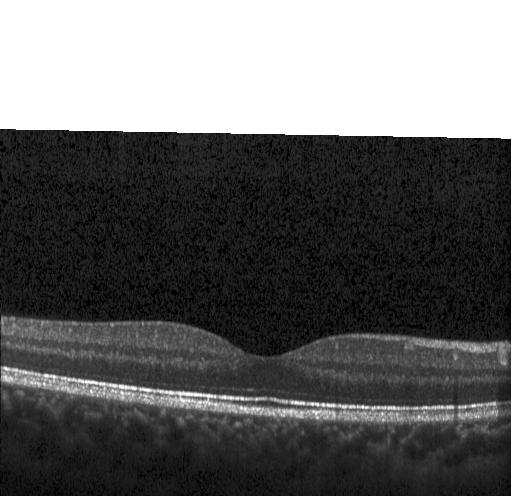 Retinal OCT cross-section.
OCT finding: neither choroidal neovascularization, diabetic macular edema, nor drusen.